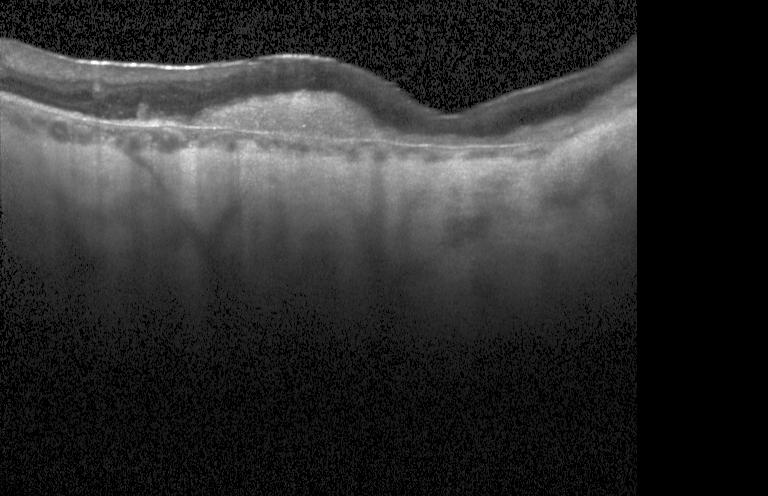 Optical coherence tomography B-scan. SD-OCT
Finding: choroidal neovascularization.